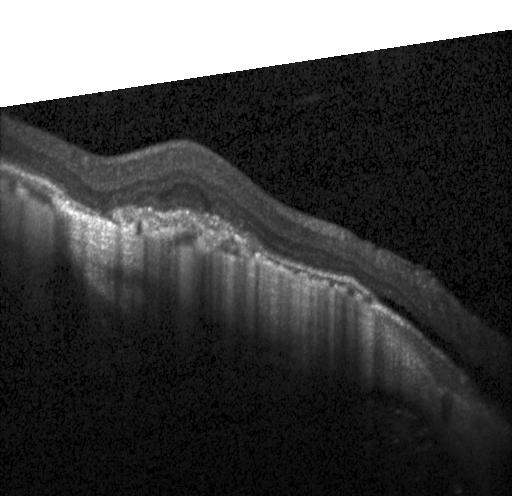 Impression: a choroidal neovascular membrane.